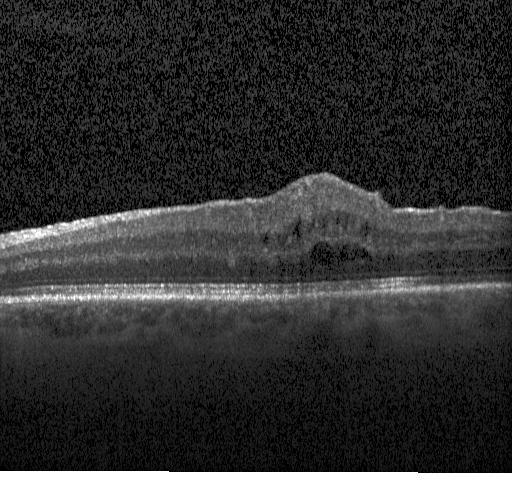

OCT finding: diabetic macular edema (DME).